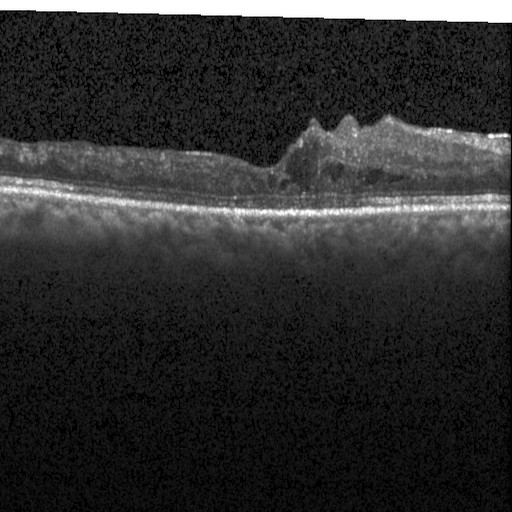
OCT B-scan showing DME.